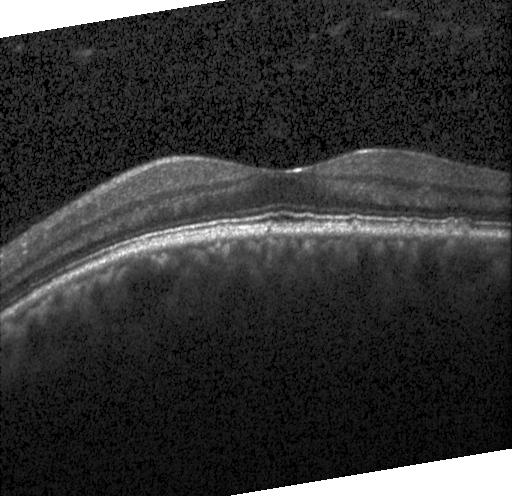 Retinal OCT cross-section showing multiple drusen.